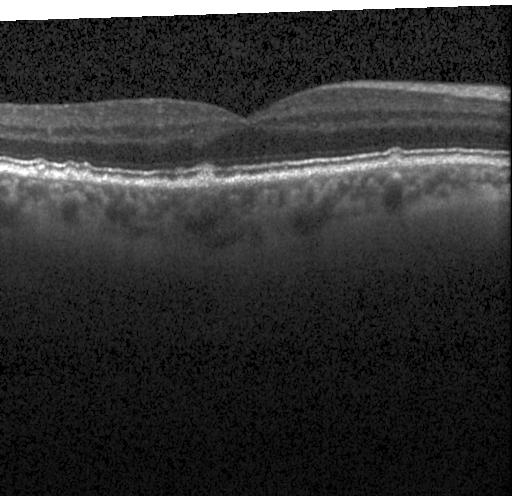 Impression: drusen.